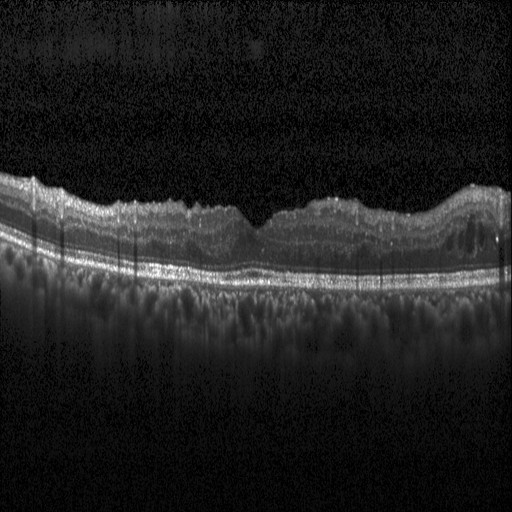 Heidelberg Spectralis OCT system. OCT B-scan. Through the macula.
Impression: diabetic macular edema (DME).